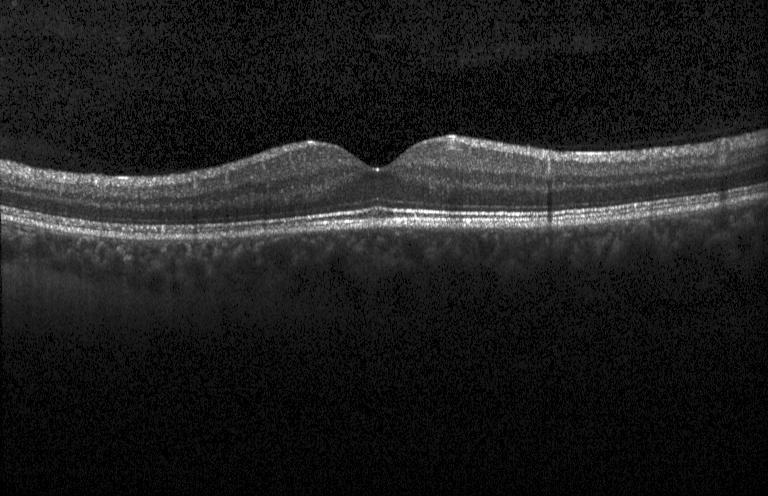

OCT finding: no choroidal neovascularization, diabetic macular edema, or drusen.